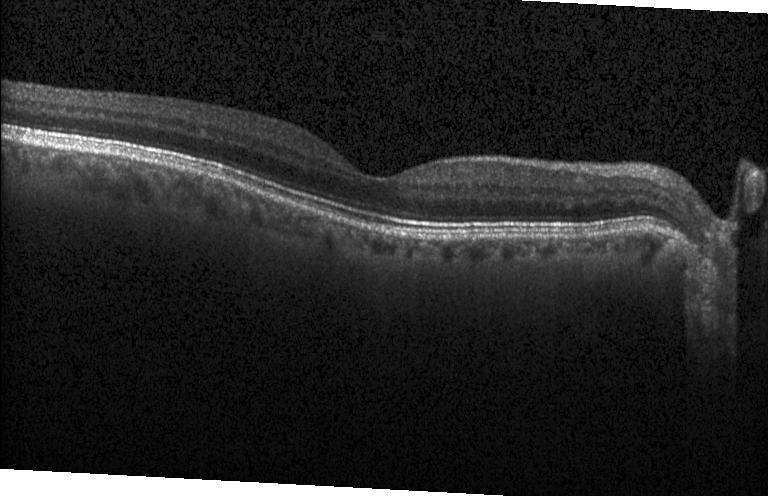 OCT B-scan; Heidelberg Spectralis. Impression: neither CNV, DME, nor drusen.